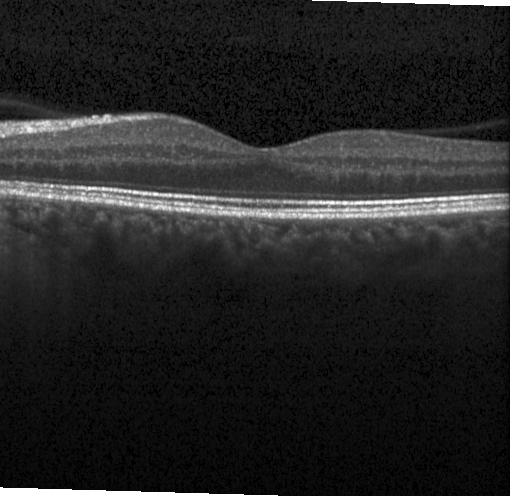
Optical coherence tomography scan · acquired on a Heidelberg Spectralis · SD-OCT · centered on the fovea. Impression: no CNV, no DME, and no drusen.